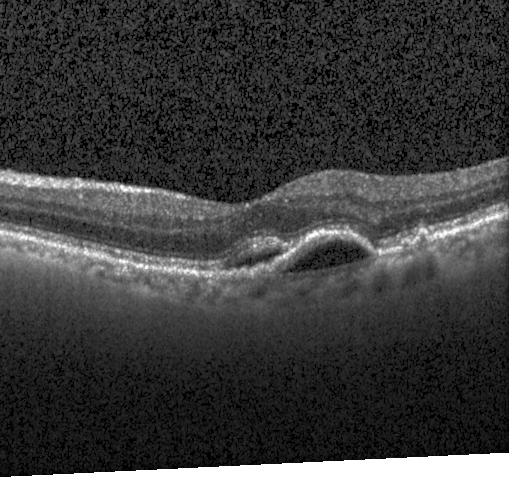 Acquired on a Heidelberg Spectralis. Spectral-domain OCT. Retinal OCT B-scan
Impression: CNV.